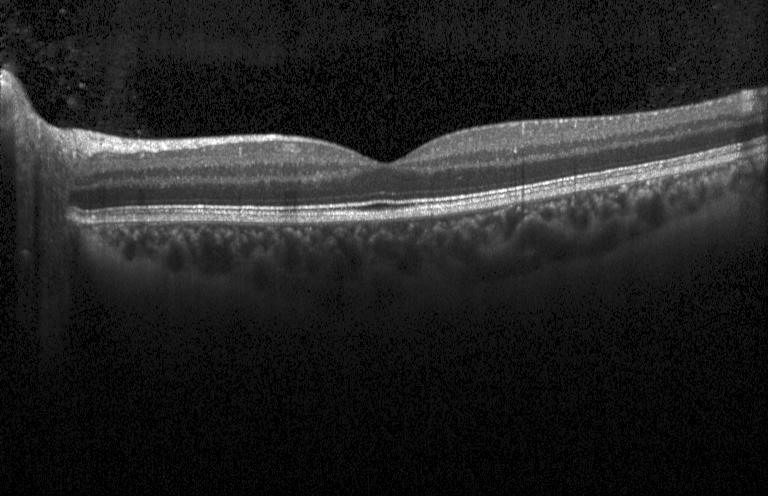 OCT line scan — Diagnosis: no CNV, DME, or drusen.